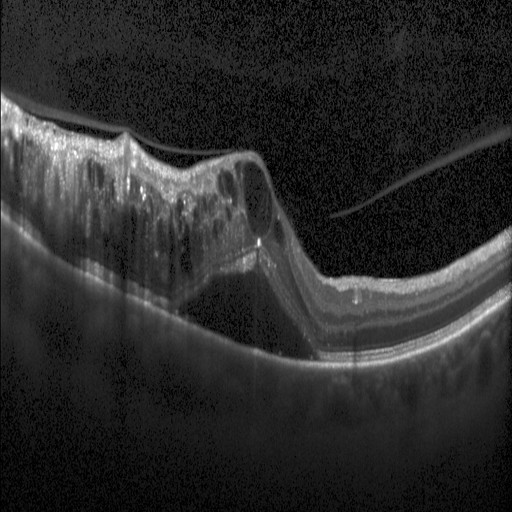

The scan shows DME.